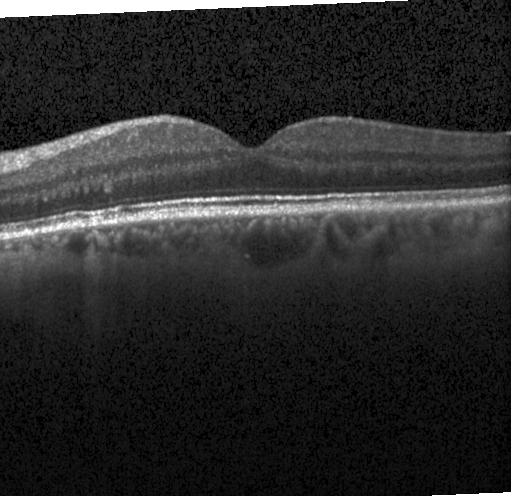

Finding: no evidence of CNV, DME, or drusen.